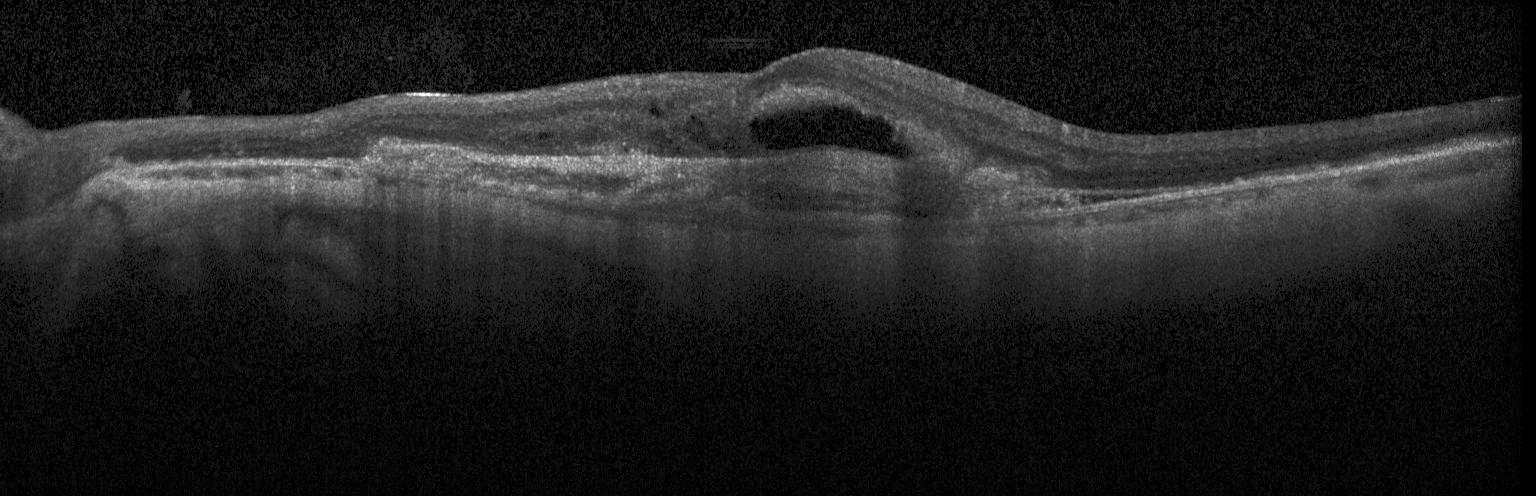 Optical coherence tomography B-scan; fovea-centered; Heidelberg Spectralis — This B-scan demonstrates CNV.